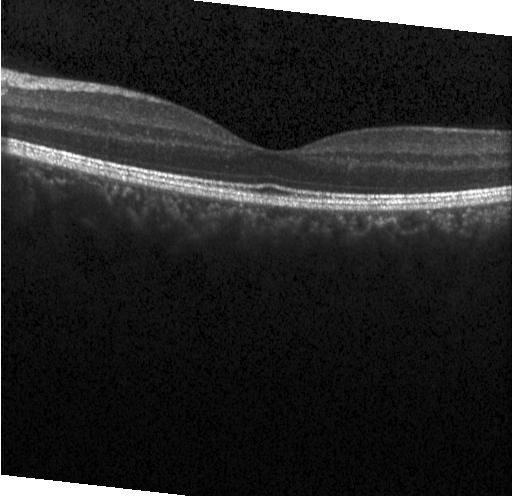
Optical coherence tomography B-scan; macular scan; SD-OCT; instrument: Heidelberg Spectralis
The scan shows no evidence of choroidal neovascularization, diabetic macular edema, or drusen.